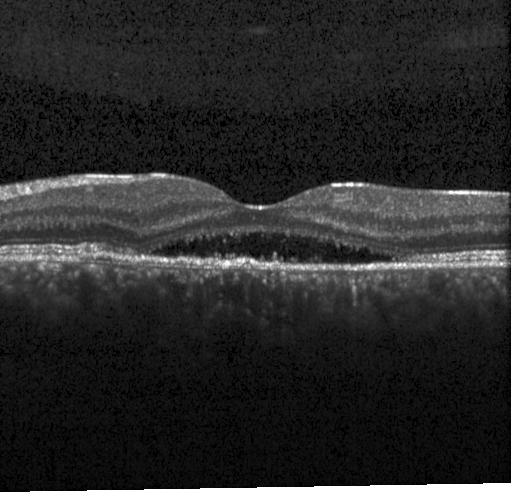

Retinal OCT cross-section · through the macula. Assessment: choroidal neovascularization (CNV).